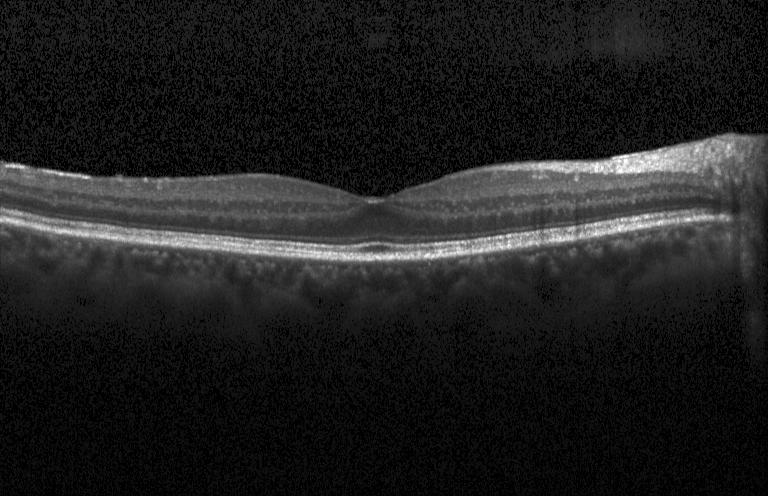
SD-OCT · Heidelberg Spectralis · OCT line scan — This B-scan demonstrates no choroidal neovascularization, no diabetic macular edema, and no drusen.